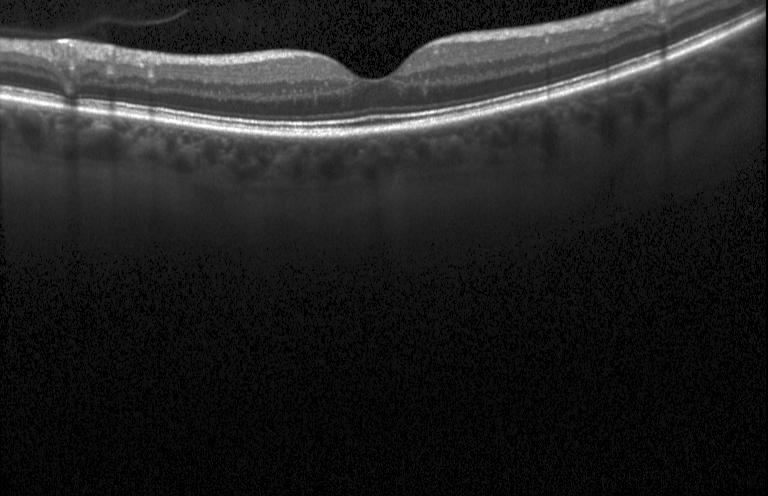 Diagnosis: no CNV, DME, or drusen.